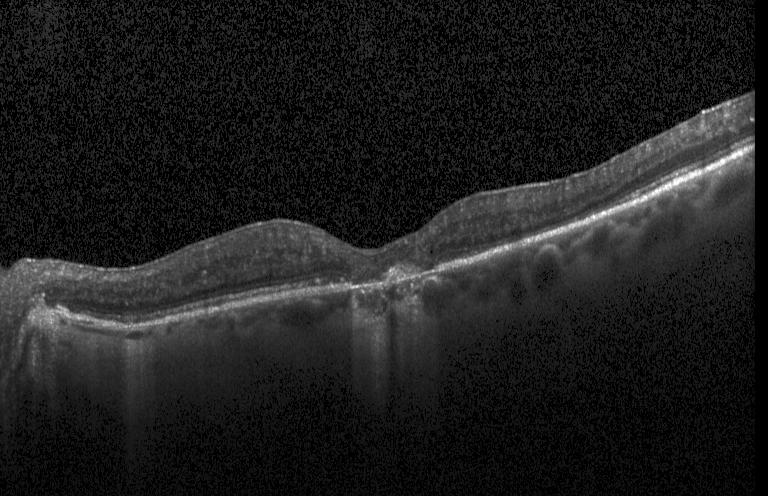

SD-OCT; OCT line scan — Impression: choroidal neovascularization.